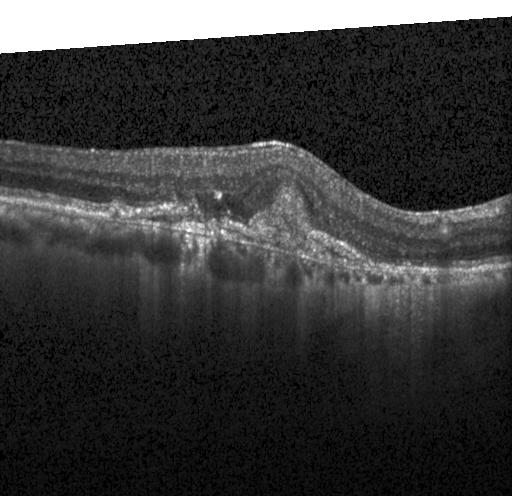
Retinal OCT cross-section · macular scan · Heidelberg Spectralis OCT system. This B-scan demonstrates a choroidal neovascular membrane.